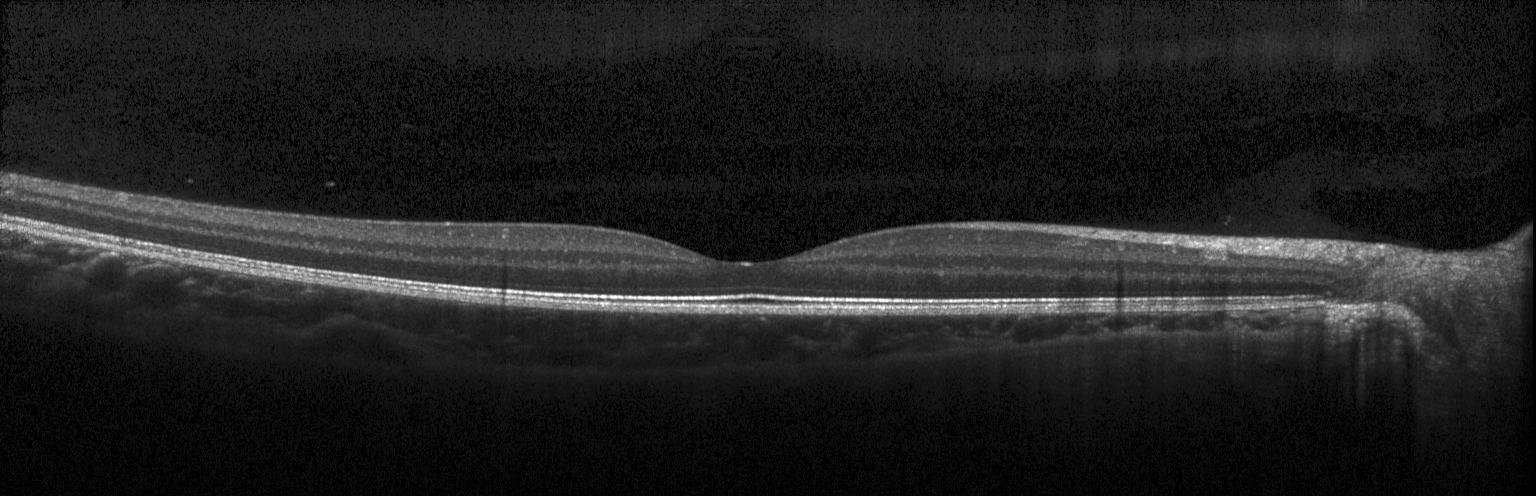

OCT B-scan — Impression: neither choroidal neovascularization, diabetic macular edema, nor drusen.